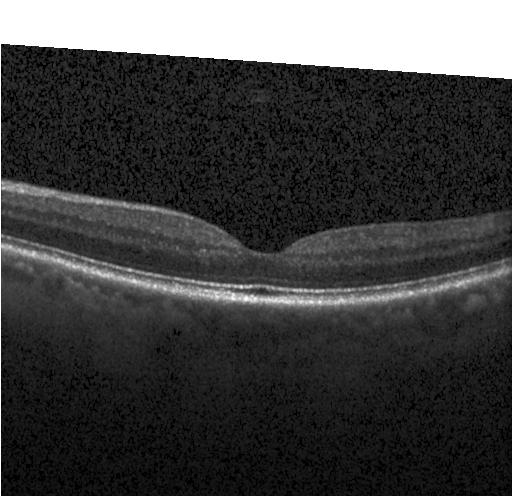 Macular OCT demonstrating neither choroidal neovascularization, diabetic macular edema, nor drusen.